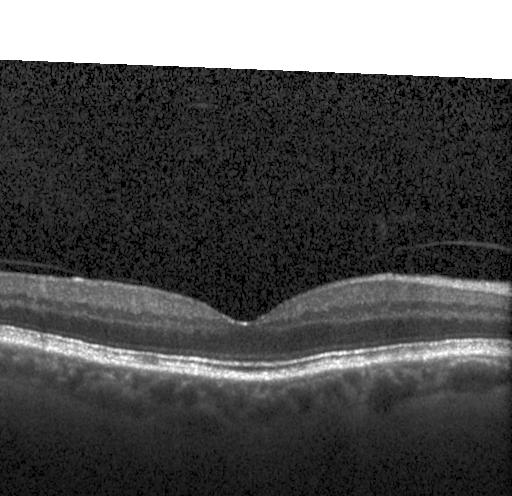 Fovea-centered. Acquired on a Heidelberg Spectralis. Optical coherence tomography B-scan
Diagnosis: no choroidal neovascularization, diabetic macular edema, or drusen.